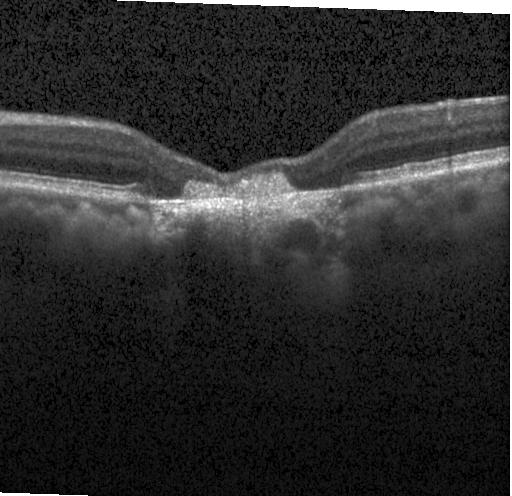 OCT B-scan, spectral-domain optical coherence tomography — Assessment: CNV.